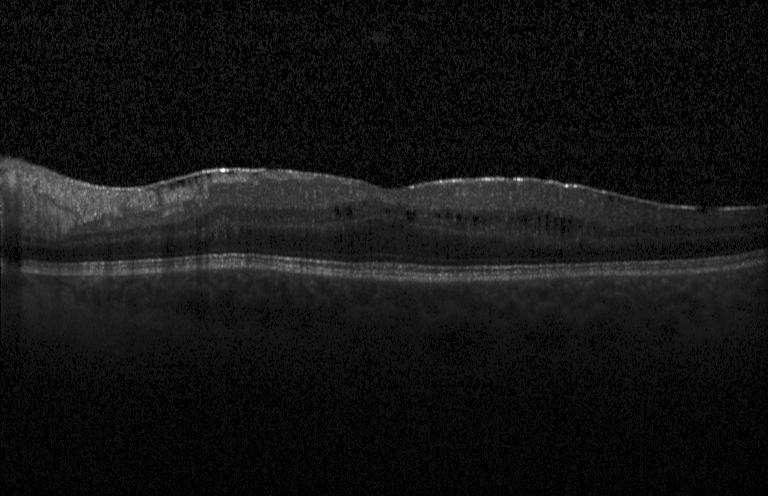

Diagnosis: diabetic macular edema.